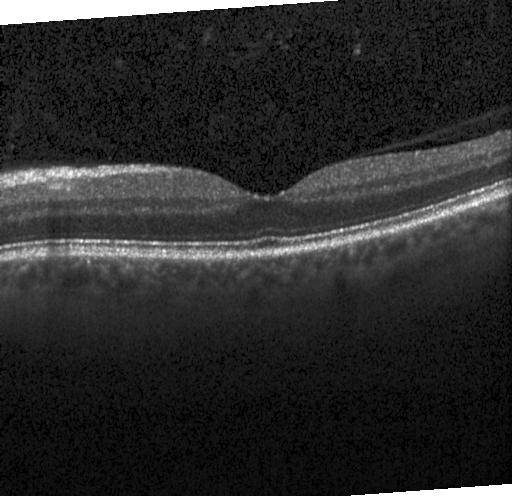
Retinal OCT cross-section
The scan shows no choroidal neovascularization, no diabetic macular edema, and no drusen.